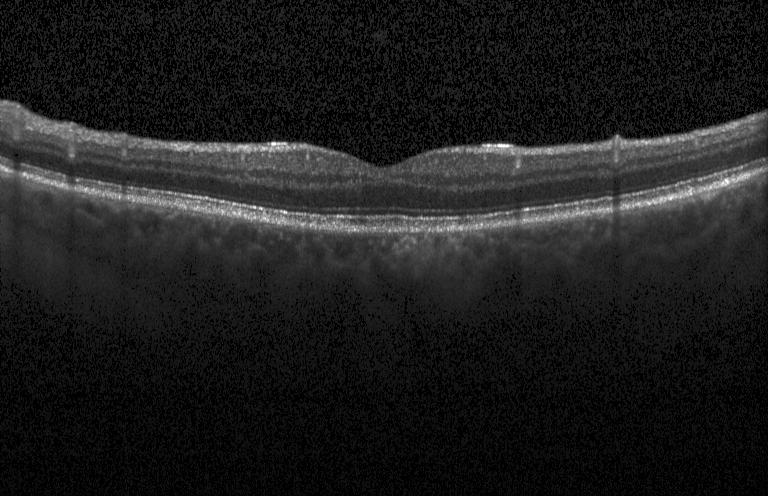 Through the macula; OCT line scan
Diagnosis: no choroidal neovascularization, no diabetic macular edema, and no drusen.